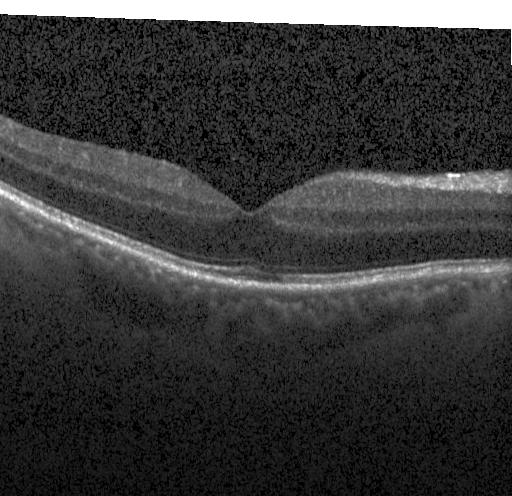

OCT line scan · acquired on a Heidelberg Spectralis · spectral-domain optical coherence tomography · horizontal scan through the fovea.
Diagnosis: no choroidal neovascularization, no diabetic macular edema, and no drusen.